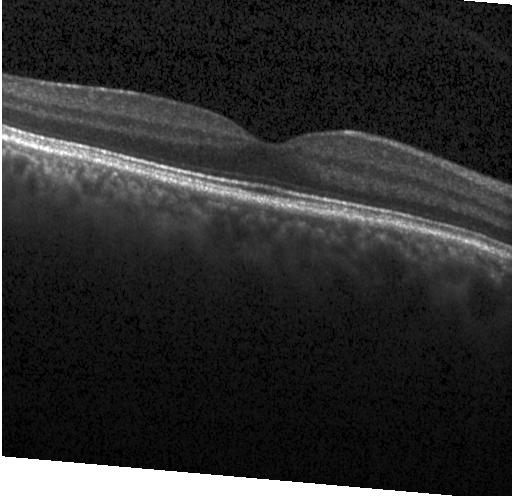
Spectral-domain optical coherence tomography. Retinal OCT B-scan. Horizontal scan through the fovea. Impression: no CNV, no DME, and no drusen.